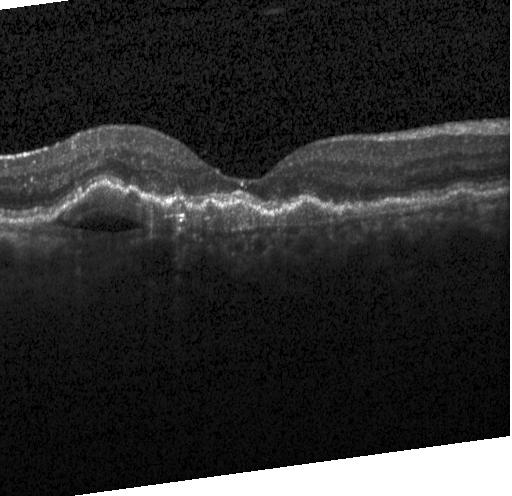 Heidelberg Spectralis. OCT line scan. SD-OCT — Assessment: a choroidal neovascular membrane.